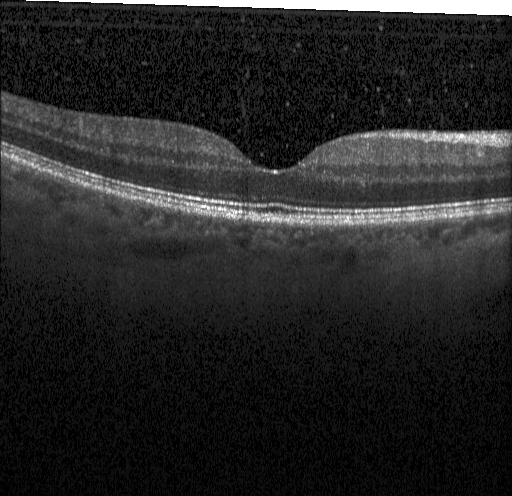

Retinal OCT B-scan; centered on the fovea; spectral-domain optical coherence tomography. No choroidal neovascularization, no diabetic macular edema, and no drusen.